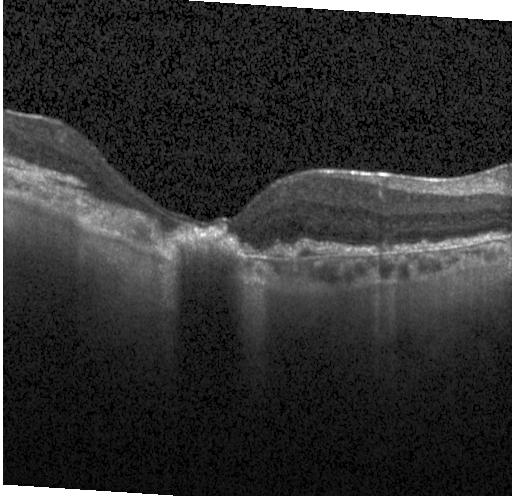
Centered on the fovea. Heidelberg Spectralis. Optical coherence tomography scan
Assessment: choroidal neovascularization (CNV).